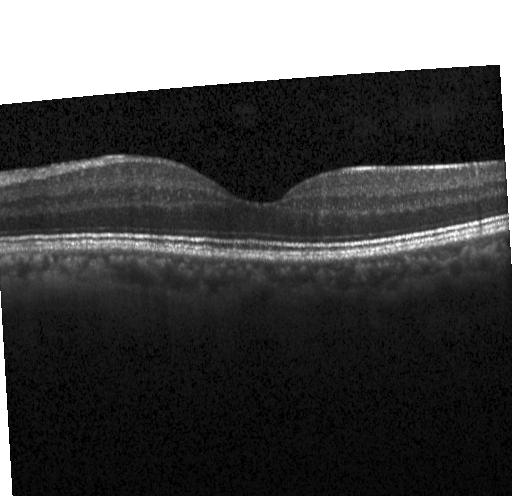
OCT scan showing no choroidal neovascularization, no diabetic macular edema, and no drusen.